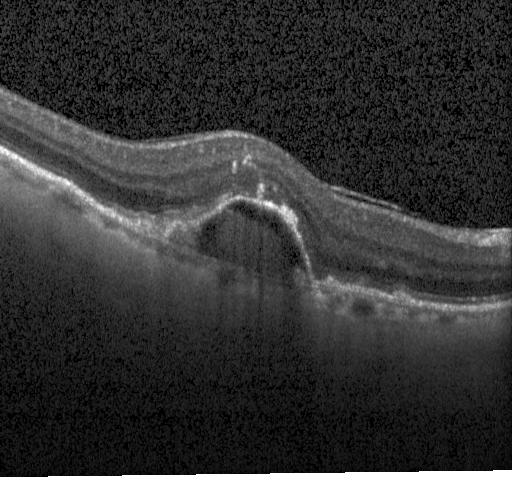

Diagnosis: a choroidal neovascular membrane.